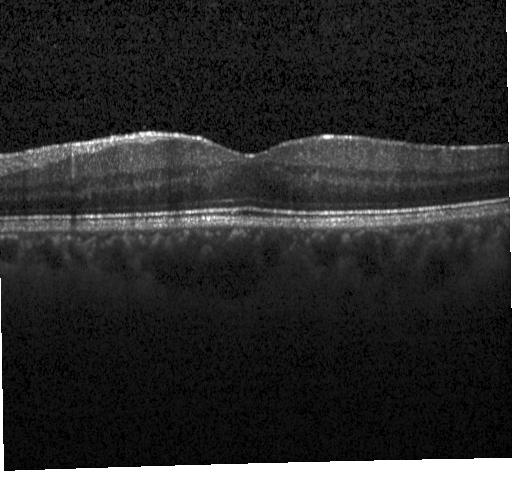

Retinal OCT B-scan, instrument: Heidelberg Spectralis, spectral-domain optical coherence tomography, centered on the fovea. Macular OCT: no choroidal neovascularization, no diabetic macular edema, and no drusen.